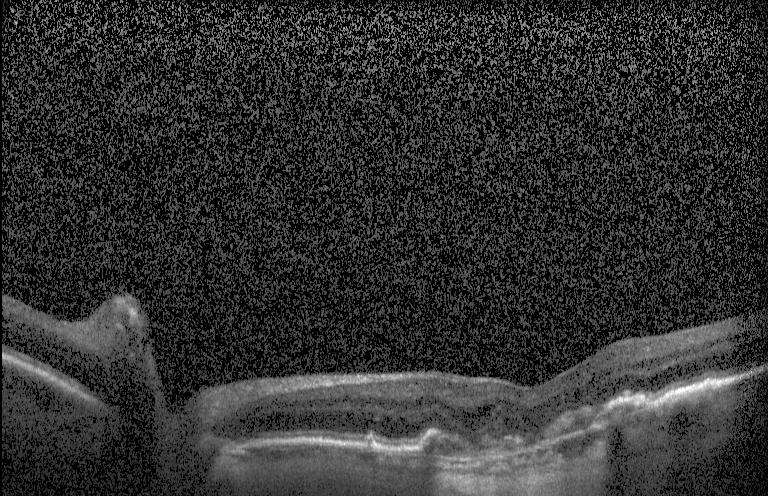 OCT line scan, acquired on a Heidelberg Spectralis, horizontal scan through the fovea — The scan shows a choroidal neovascular membrane.